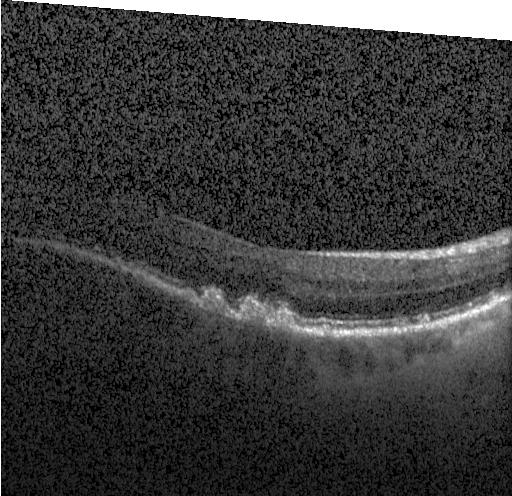 Retinal OCT cross-section, fovea-centered, Heidelberg Spectralis OCT system, spectral-domain optical coherence tomography. Assessment: sub-RPE drusenoid deposits.